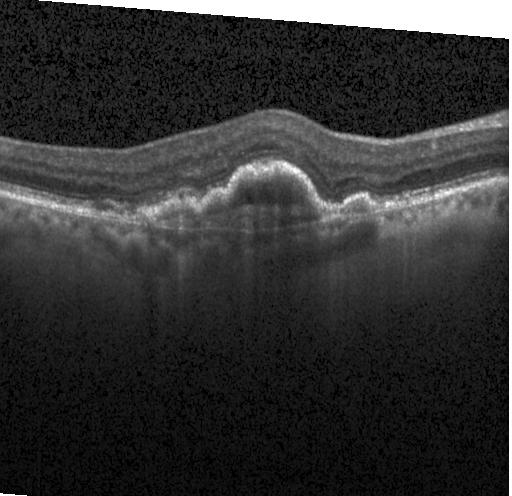
Macular OCT: a choroidal neovascular membrane.